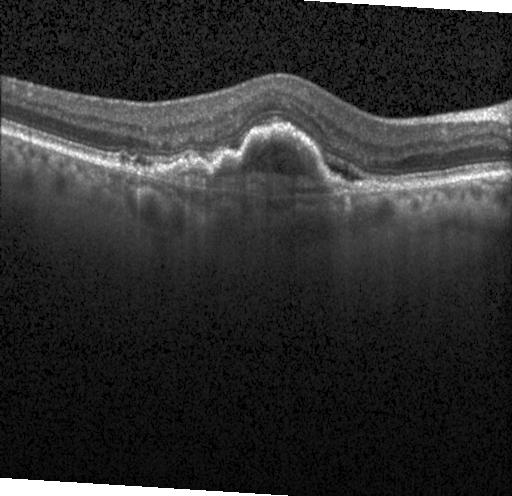 Optical coherence tomography B-scan — The scan shows choroidal neovascularization (CNV).